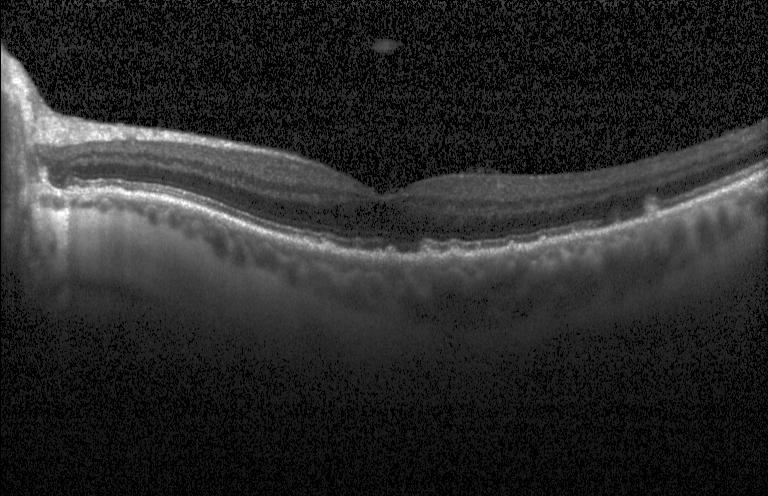 Diagnosis: drusen.